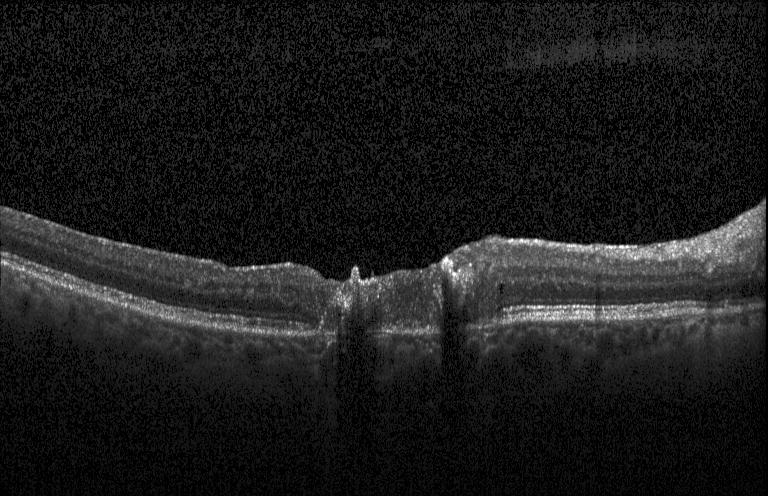 Retinal OCT cross-section. Heidelberg Spectralis OCT system. Fovea-centered. SD-OCT
A choroidal neovascular membrane.